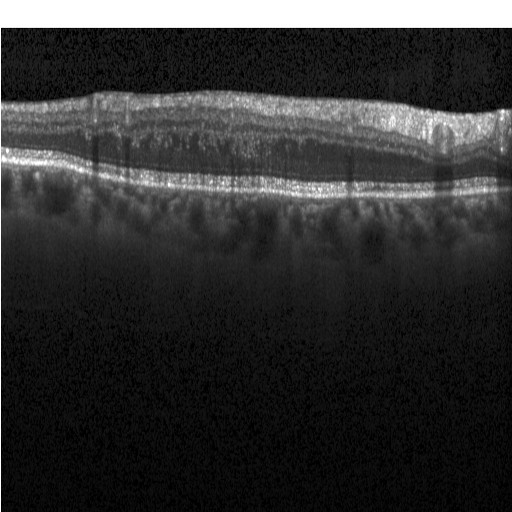
Instrument: Heidelberg Spectralis; OCT B-scan
Diagnosis: diabetic macular edema.